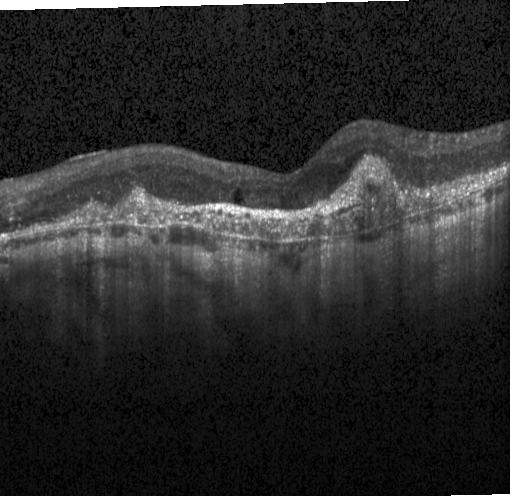

Retinal OCT B-scan, fovea-centered — Finding: choroidal neovascularization.